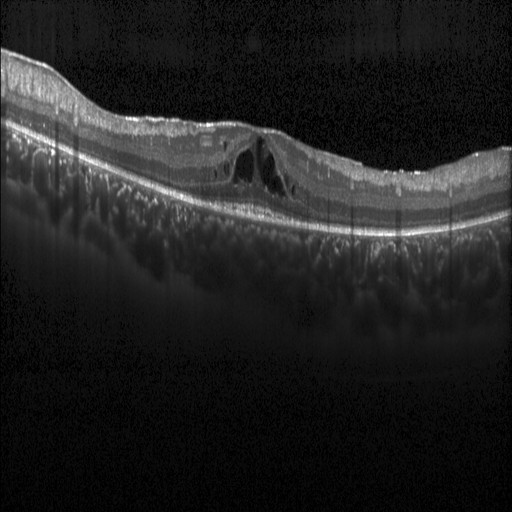 Optical coherence tomography scan.
DME.